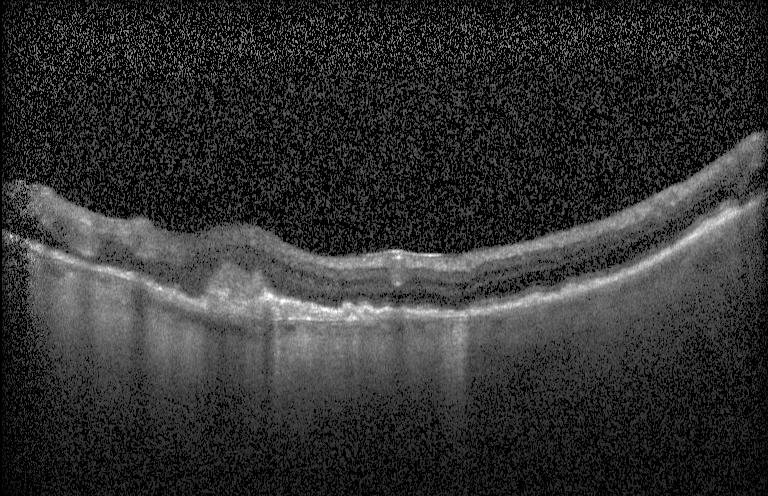

OCT finding: a choroidal neovascular membrane.